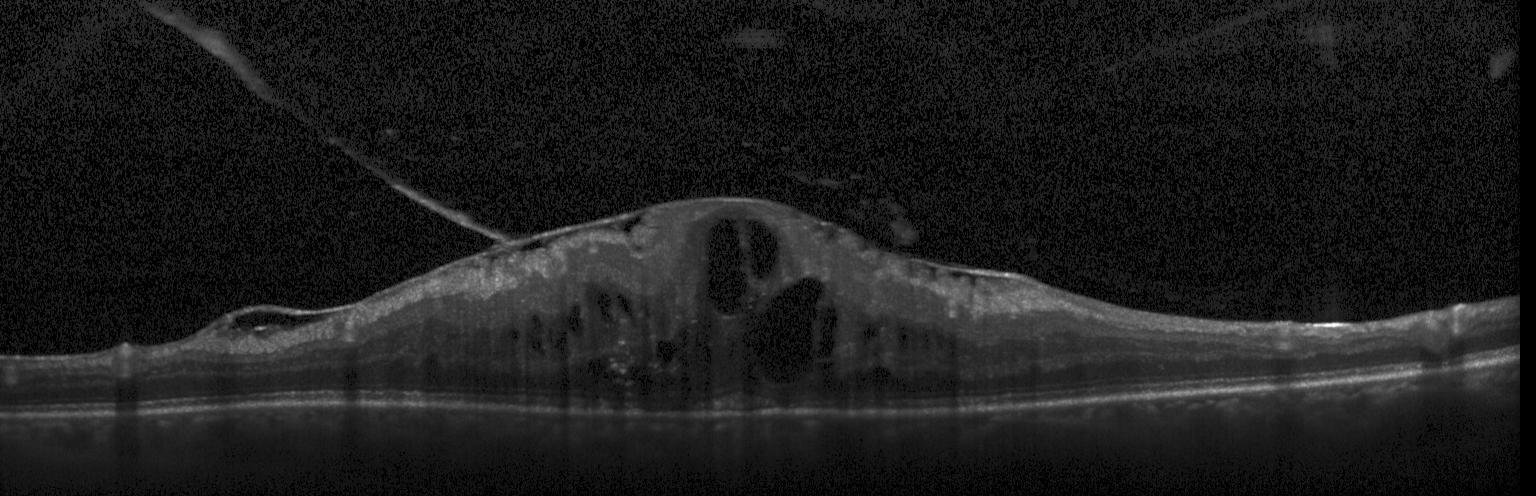
OCT B-scan showing DME.